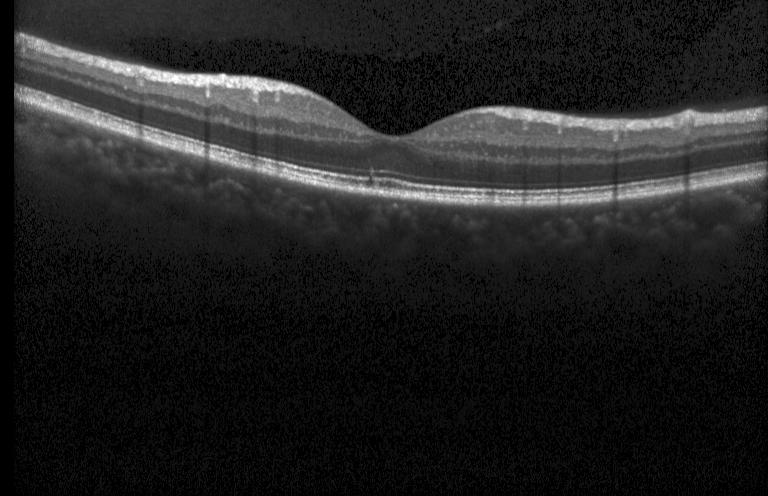 Retinal OCT B-scan · through the macula · spectral-domain optical coherence tomography. This B-scan demonstrates no choroidal neovascularization, no diabetic macular edema, and no drusen.